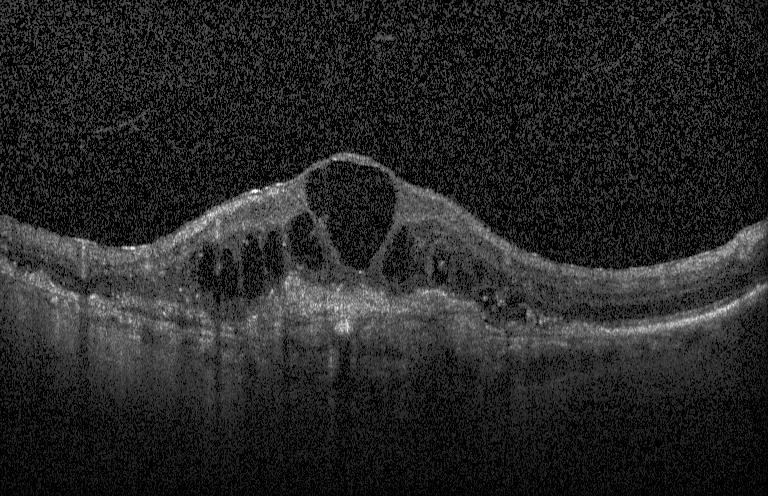

Acquired on a Heidelberg Spectralis, retinal OCT B-scan — Finding: choroidal neovascularization (CNV).